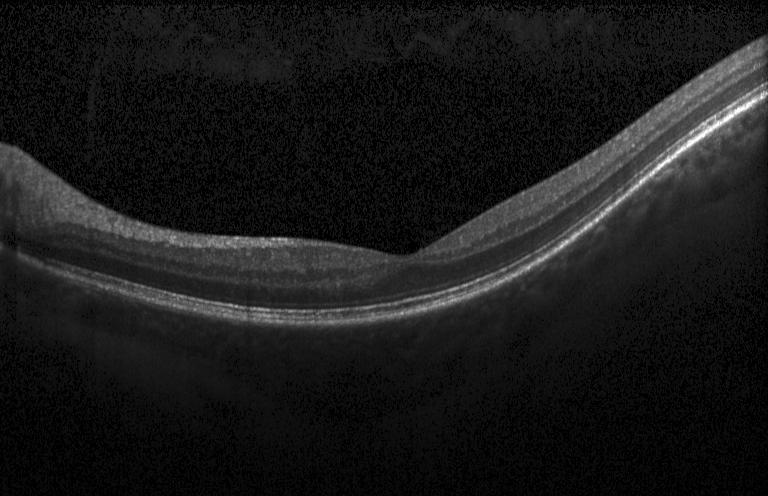 No CNV, no DME, and no drusen.